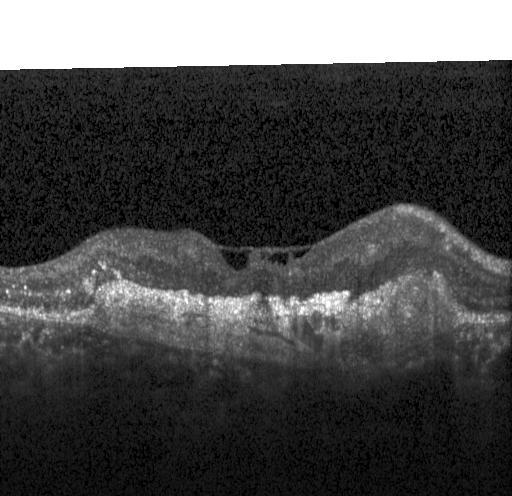 OCT B-scan showing a choroidal neovascular membrane.